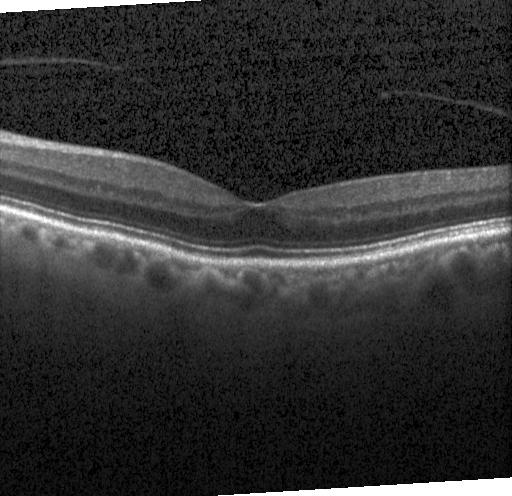

Finding: neither CNV, DME, nor drusen.